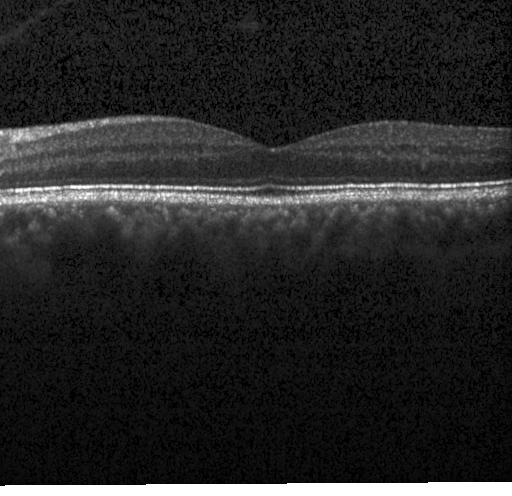
Retinal OCT cross-section. Diagnosis: no choroidal neovascularization, no diabetic macular edema, and no drusen.